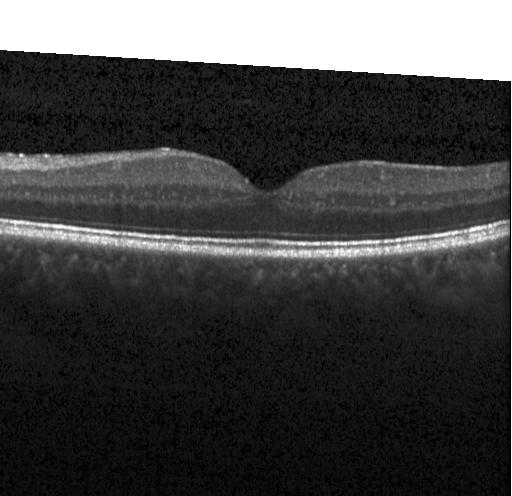
OCT B-scan · spectral-domain OCT — Diagnosis: no choroidal neovascularization, diabetic macular edema, or drusen.